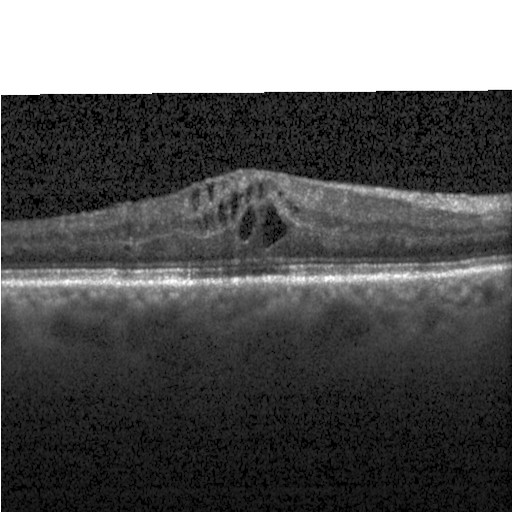
OCT B-scan showing diabetic macular edema.